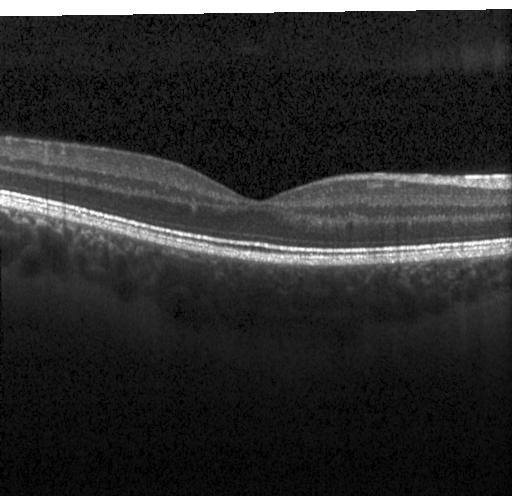 Macular scan, optical coherence tomography scan, spectral-domain OCT.
Finding: no choroidal neovascularization, diabetic macular edema, or drusen.